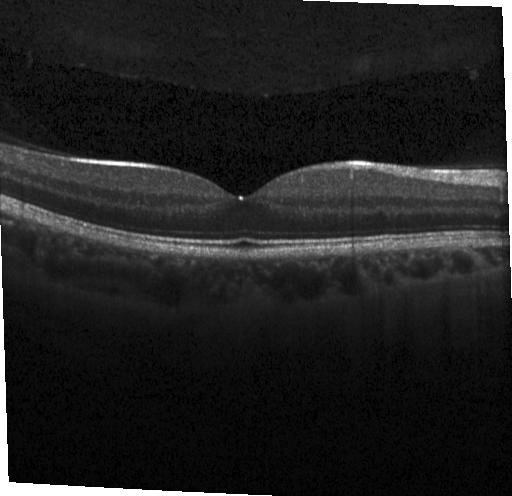 Fovea-centered. Retinal OCT B-scan
The scan shows no evidence of CNV, DME, or drusen.